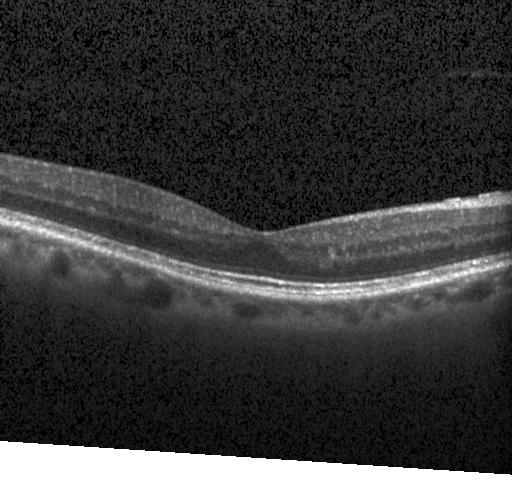

Macular scan, OCT line scan.
Diagnosis: no choroidal neovascularization, no diabetic macular edema, and no drusen.